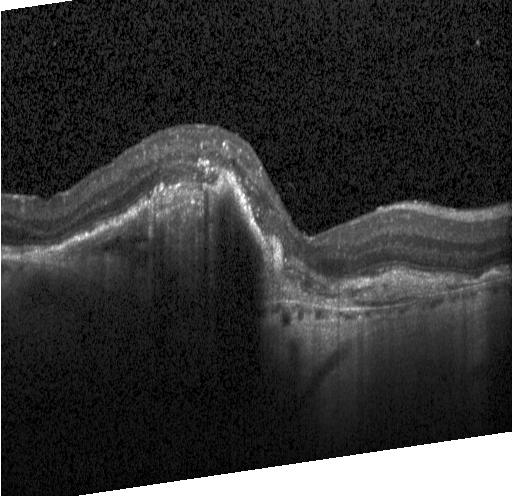

OCT B-scan showing a choroidal neovascular membrane.